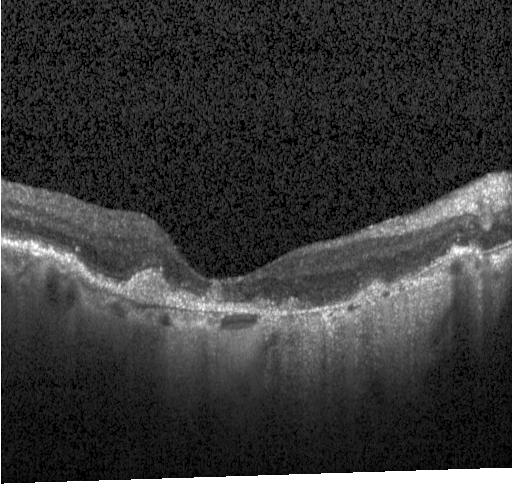 Macular OCT: choroidal neovascularization.